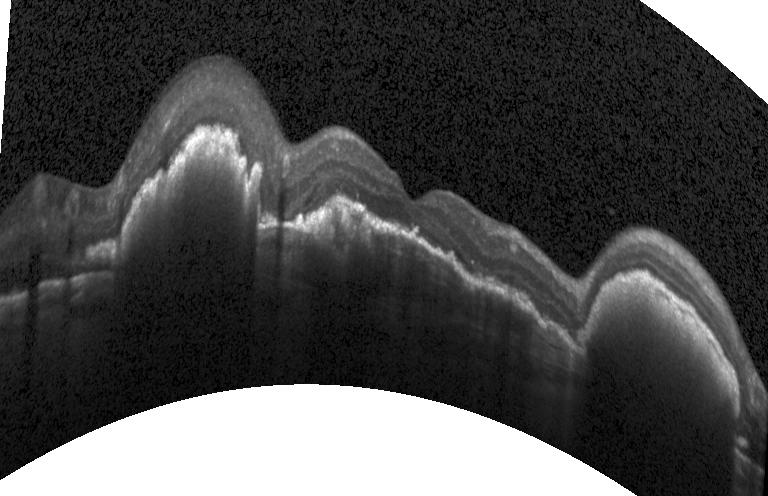

Spectral-domain OCT. Macular scan. Optical coherence tomography scan. This B-scan demonstrates a choroidal neovascular membrane.